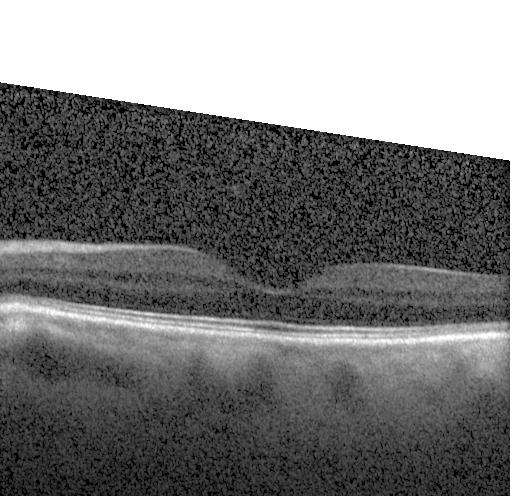

Spectral-domain OCT B-scan: no evidence of CNV, DME, or drusen.